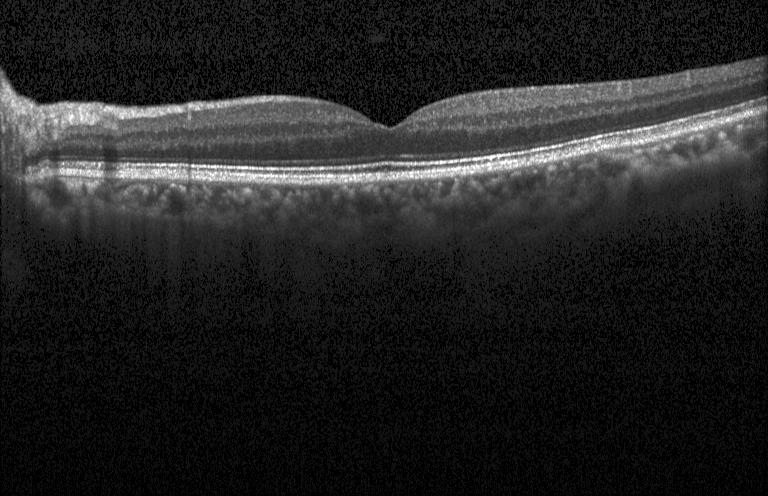

Optical coherence tomography scan, Heidelberg Spectralis OCT system
Impression: no evidence of CNV, DME, or drusen.